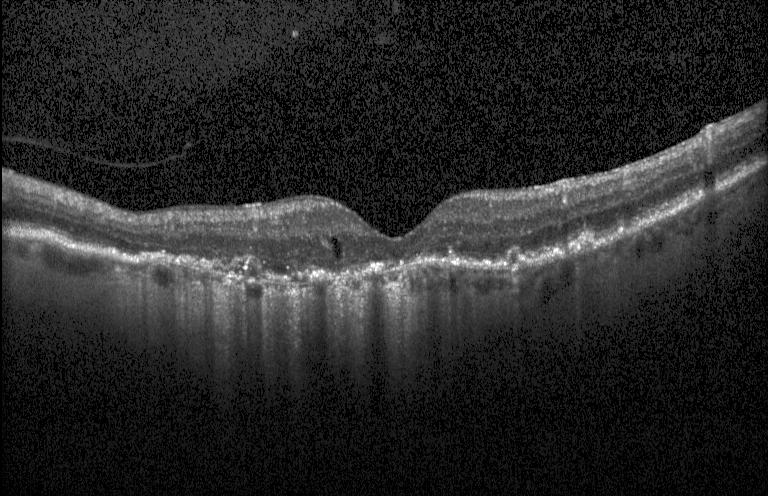

Retinal OCT B-scan. The scan shows a choroidal neovascular membrane.